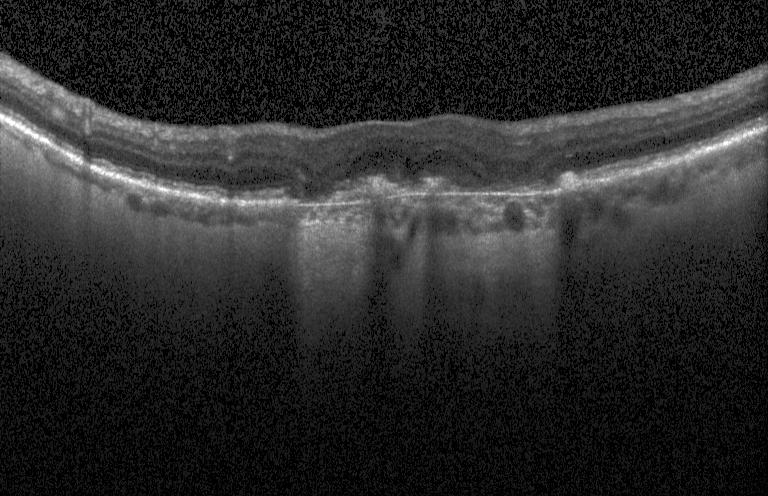

Instrument: Heidelberg Spectralis. Optical coherence tomography scan.
Assessment: a choroidal neovascular membrane.